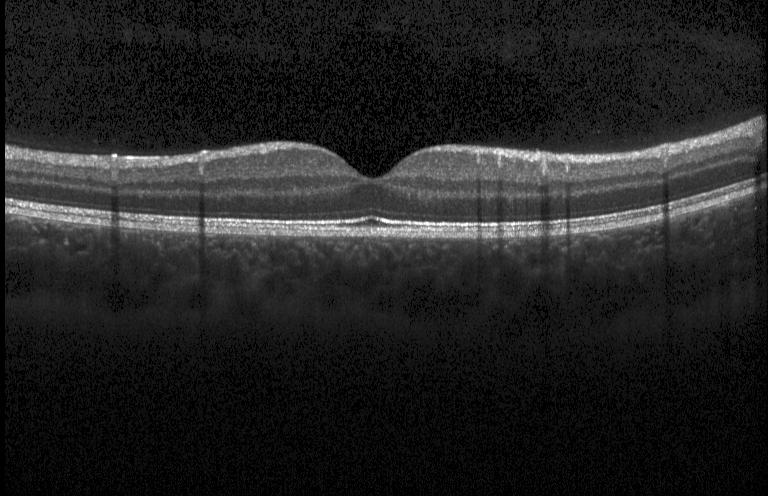
SD-OCT · fovea-centered · retinal OCT B-scan. Macular OCT: no evidence of choroidal neovascularization, diabetic macular edema, or drusen.